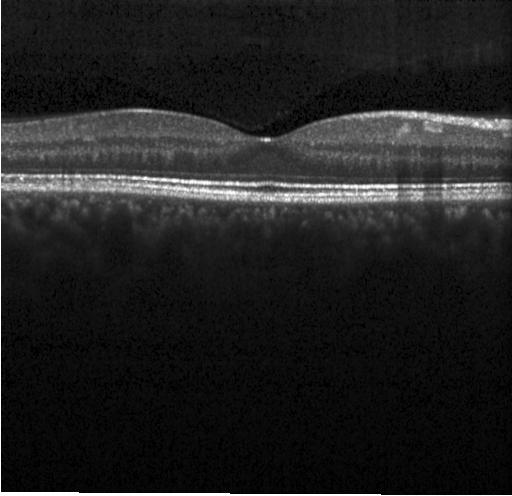

Macular OCT demonstrating no evidence of choroidal neovascularization, diabetic macular edema, or drusen.